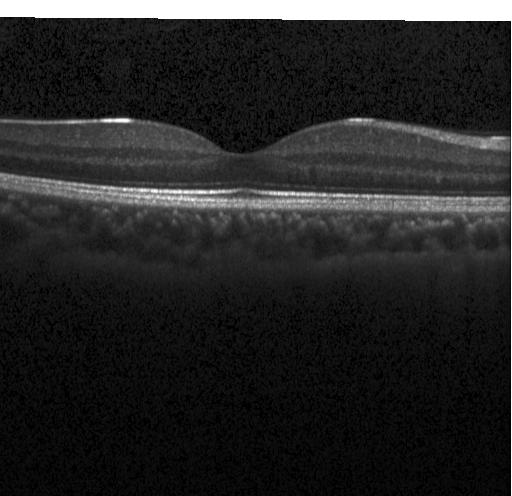 OCT line scan
Finding: no choroidal neovascularization, no diabetic macular edema, and no drusen.